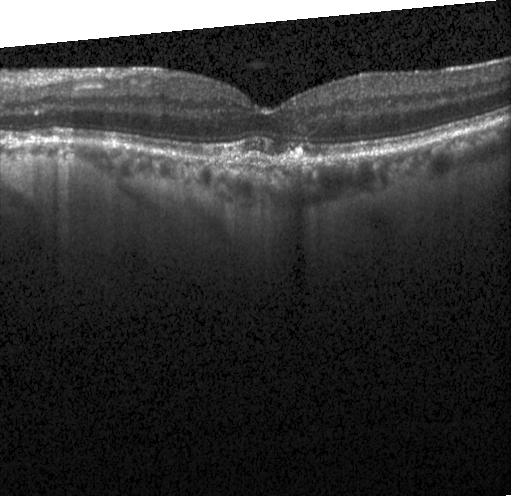

Retinal OCT B-scan.
Dx: a choroidal neovascular membrane.